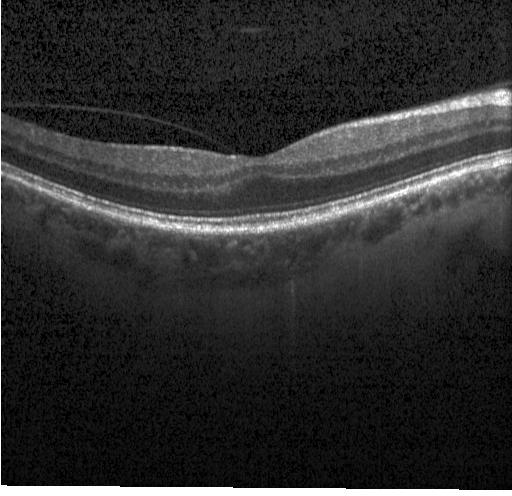
Finding: no choroidal neovascularization, no diabetic macular edema, and no drusen.